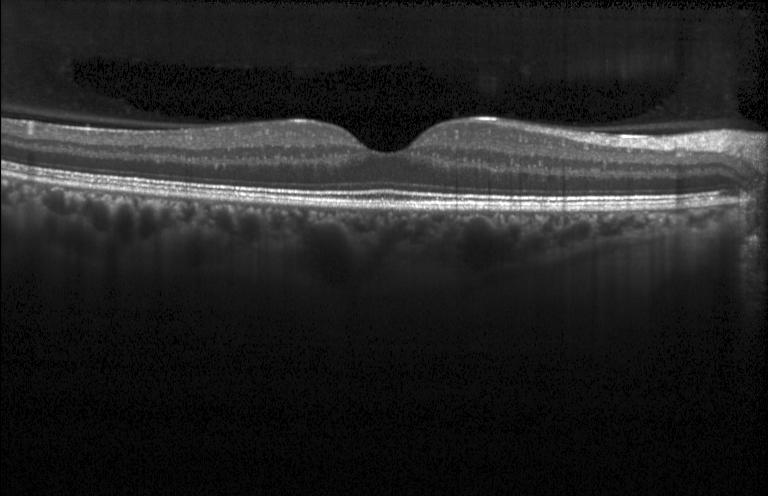

Retinal OCT cross-section. Heidelberg Spectralis
Assessment: no CNV, no DME, and no drusen.